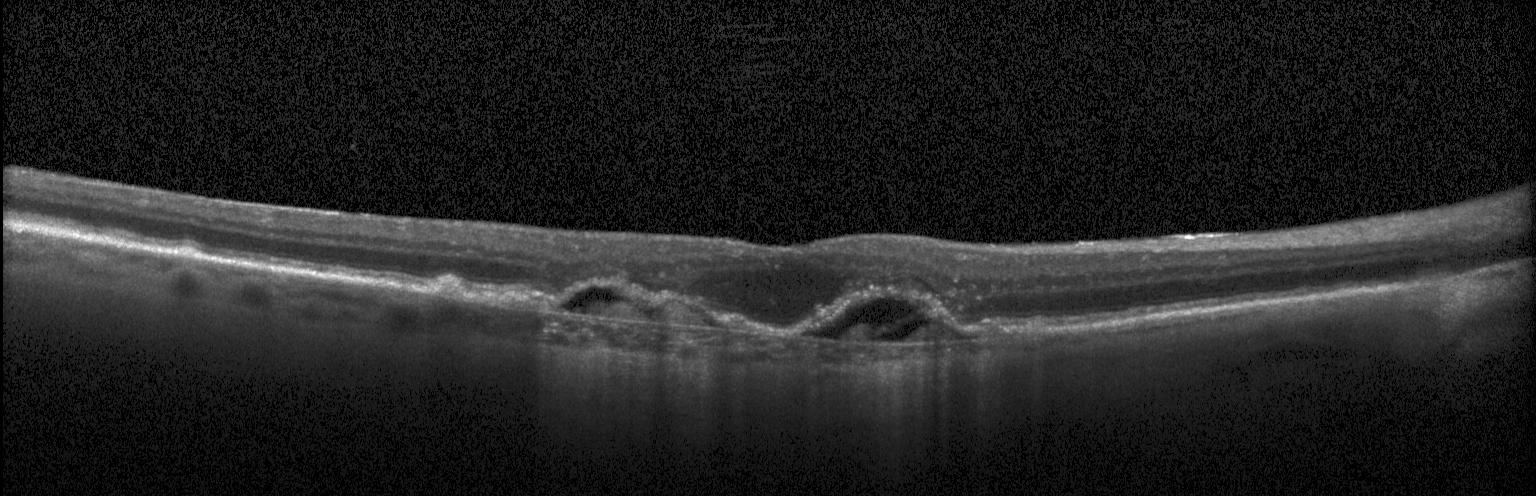

Macular OCT: choroidal neovascularization.